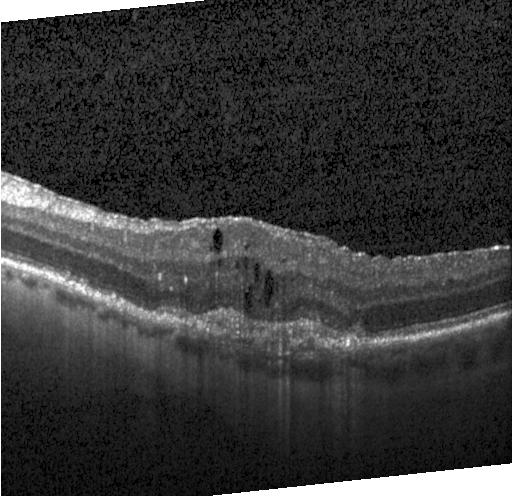
Heidelberg Spectralis OCT system. Macular scan. Retinal OCT B-scan
OCT finding: choroidal neovascularization.